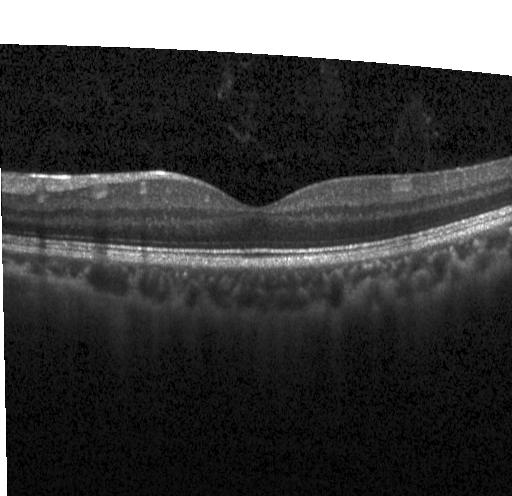
Diagnosis: neither choroidal neovascularization, diabetic macular edema, nor drusen.